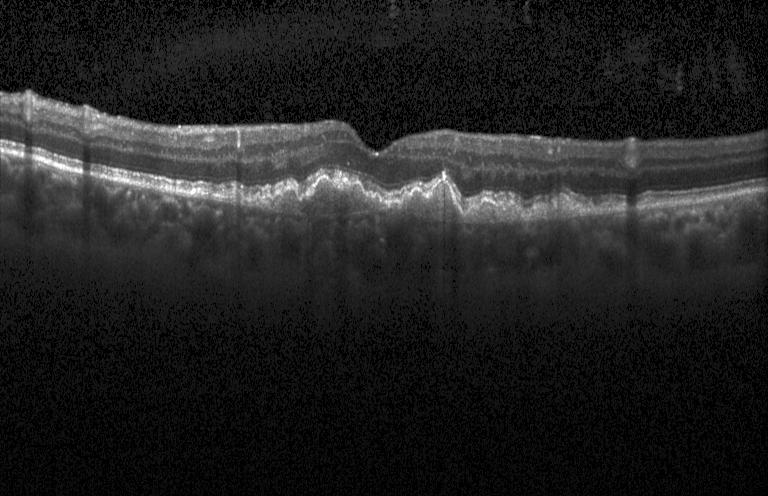
Optical coherence tomography B-scan.
Diagnosis: choroidal neovascularization (CNV).